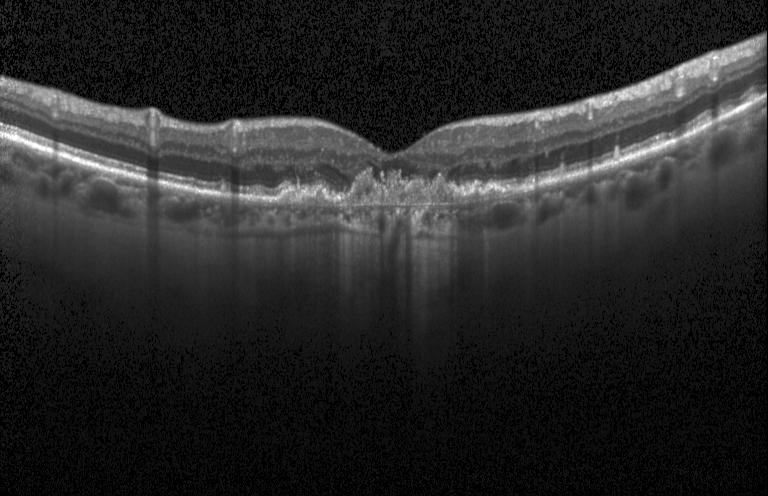

OCT line scan, SD-OCT, centered on the fovea, acquired on a Heidelberg Spectralis.
Finding: CNV.